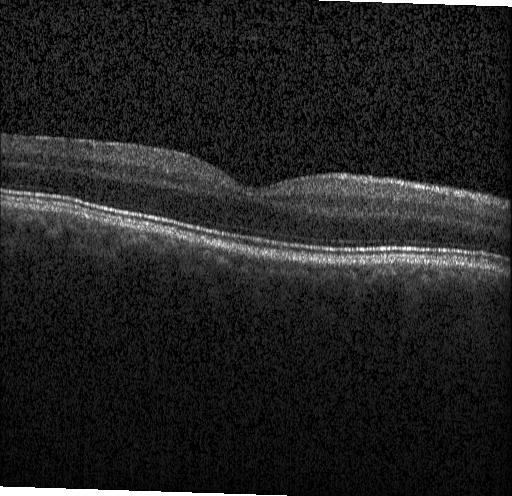

OCT B-scan showing no choroidal neovascularization, diabetic macular edema, or drusen.